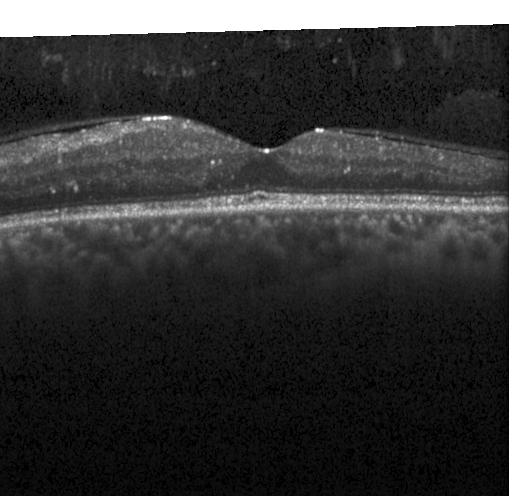

Diabetic macular edema (DME).